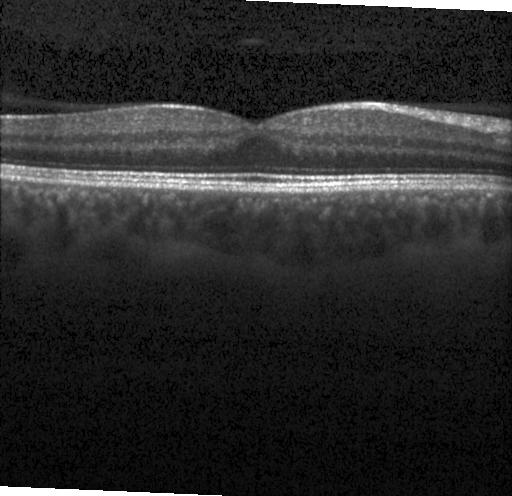
Spectral-domain OCT · optical coherence tomography scan — Macular OCT: no CNV, no DME, and no drusen.